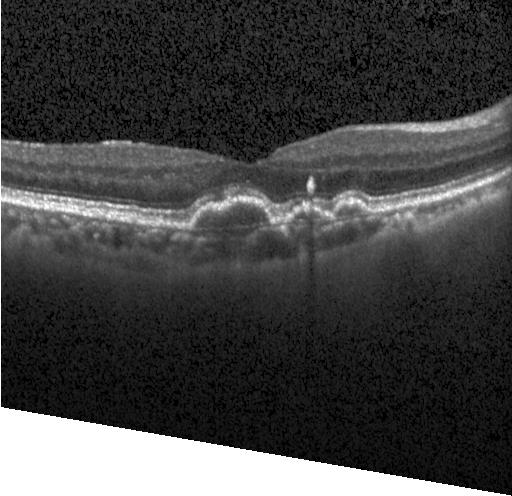

Spectral-domain OCT; OCT line scan; acquired on a Heidelberg Spectralis — Impression: choroidal neovascularization.